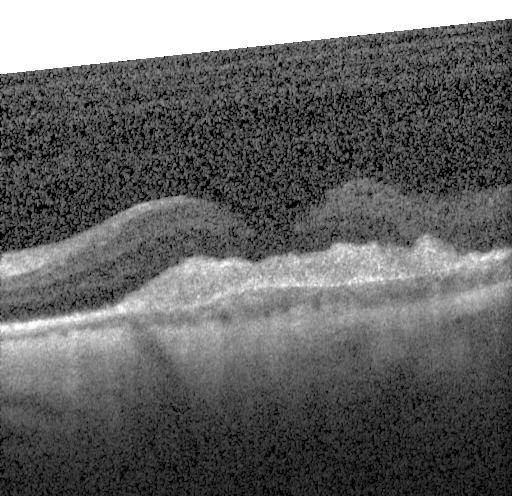
Acquired on a Heidelberg Spectralis; spectral-domain OCT; centered on the fovea; OCT B-scan — CNV.